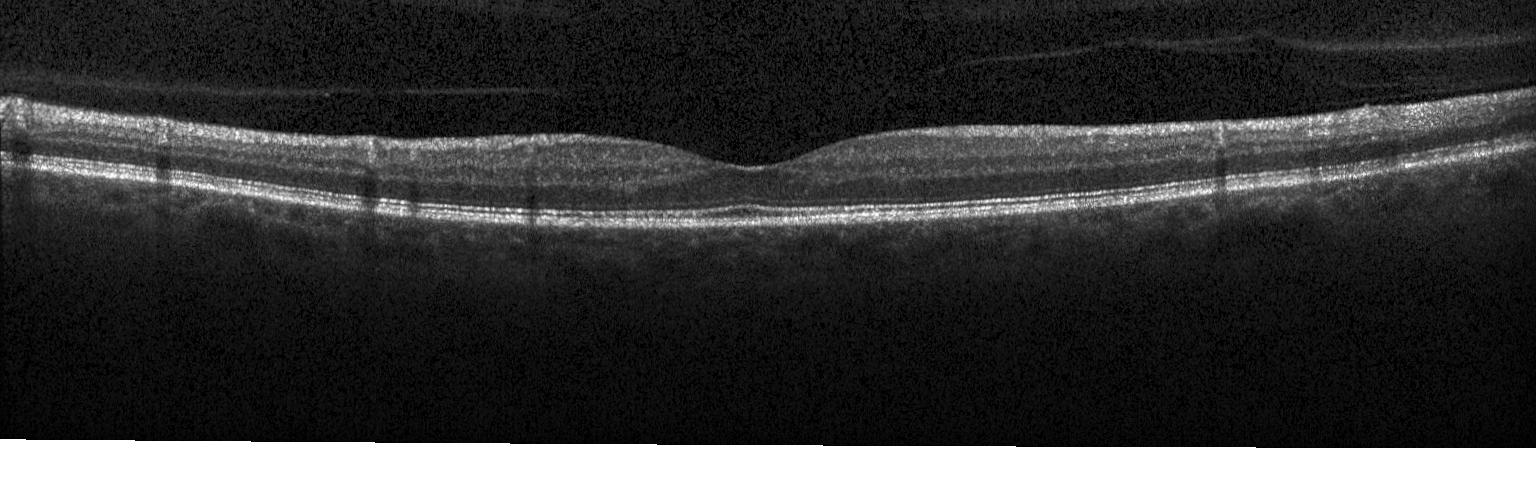

Through the macula, OCT B-scan, acquired on a Heidelberg Spectralis, spectral-domain optical coherence tomography. Impression: no choroidal neovascularization, no diabetic macular edema, and no drusen.